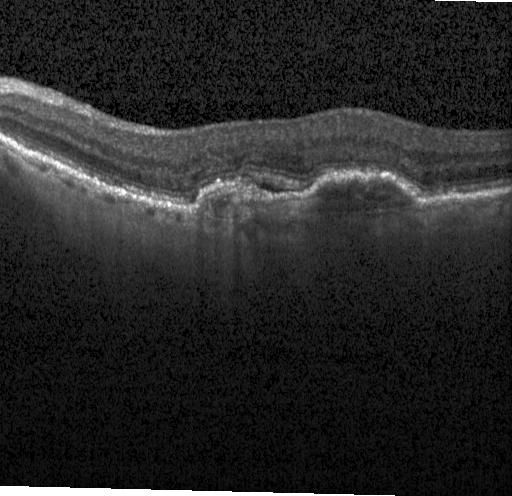

SD-OCT, fovea-centered, OCT line scan, instrument: Heidelberg Spectralis.
Impression: choroidal neovascularization.